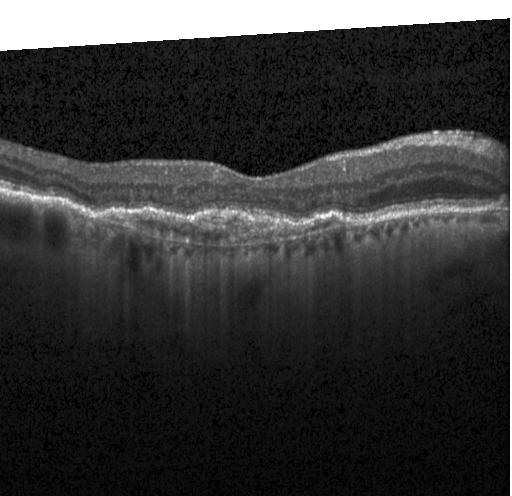

Diagnosis: choroidal neovascularization (CNV).